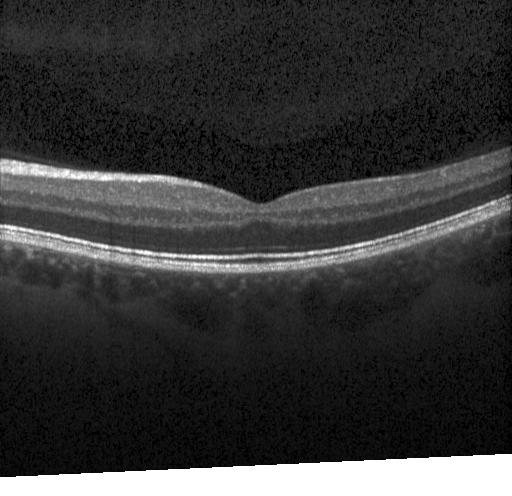

The scan shows no evidence of choroidal neovascularization, diabetic macular edema, or drusen.